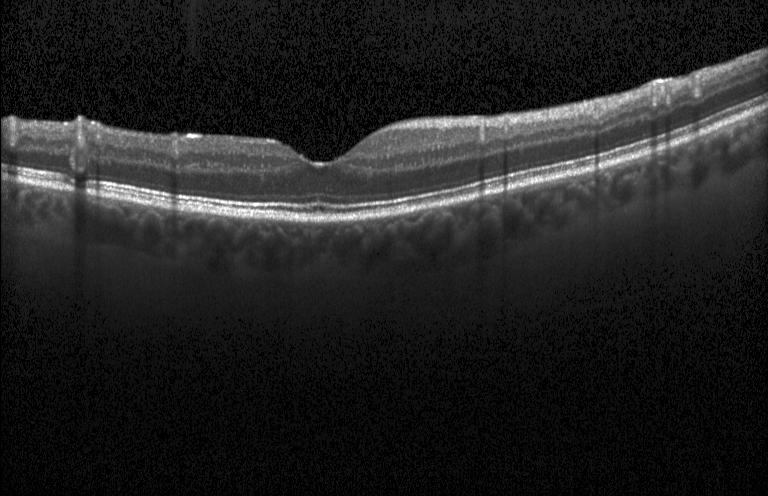 Through the macula · OCT B-scan
Finding: no evidence of choroidal neovascularization, diabetic macular edema, or drusen.